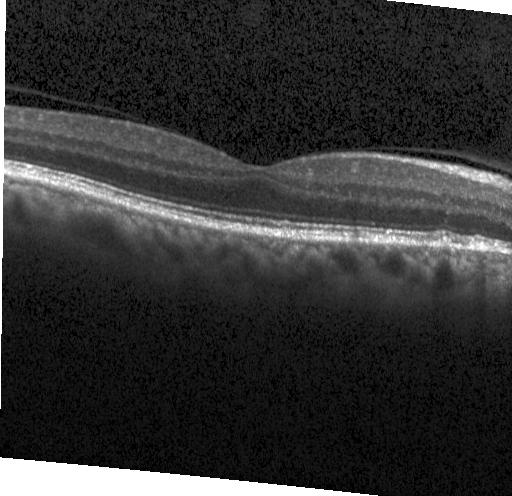 Finding: sub-RPE drusenoid deposits.